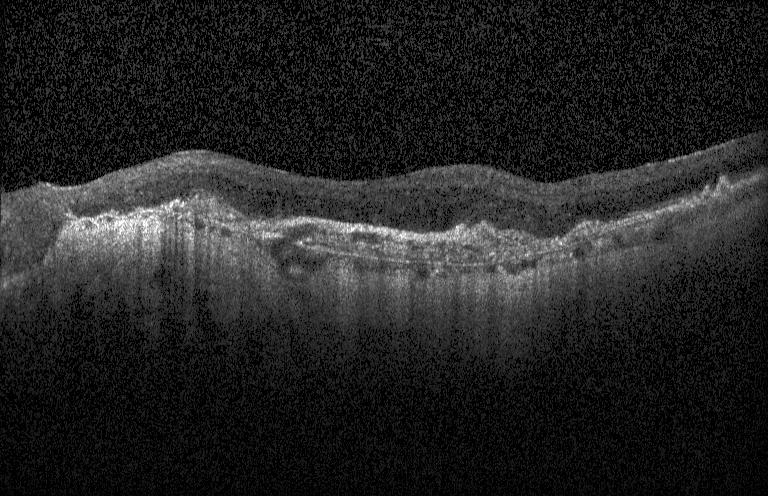
SD-OCT · optical coherence tomography B-scan. Impression: a choroidal neovascular membrane.